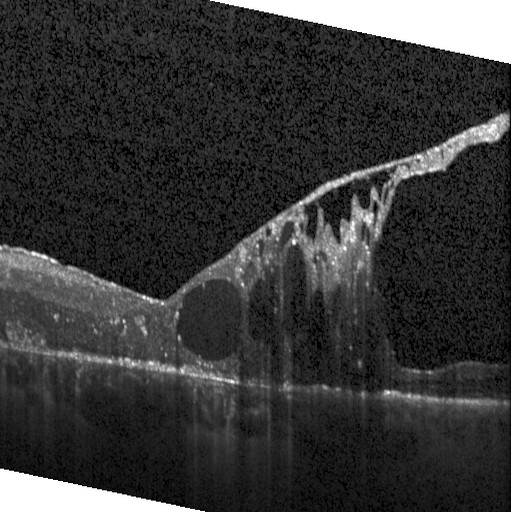 Retinal OCT cross-section showing diabetic macular edema.